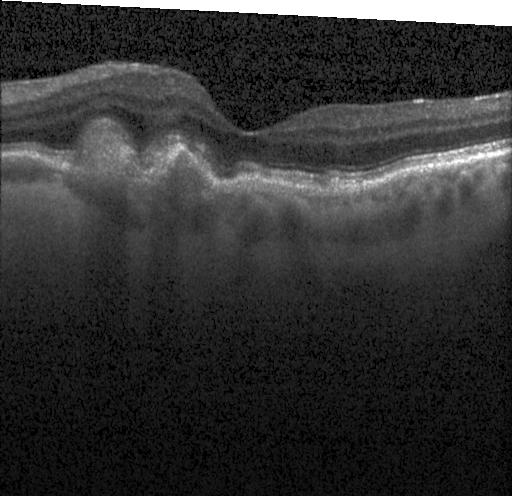

Retinal OCT B-scan.
Finding: a choroidal neovascular membrane.